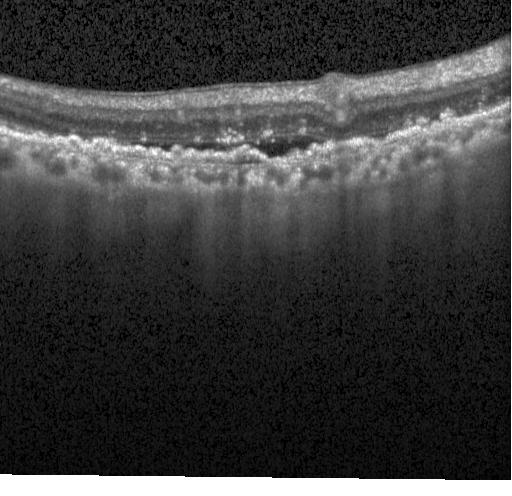

Optical coherence tomography scan — The scan shows a choroidal neovascular membrane.